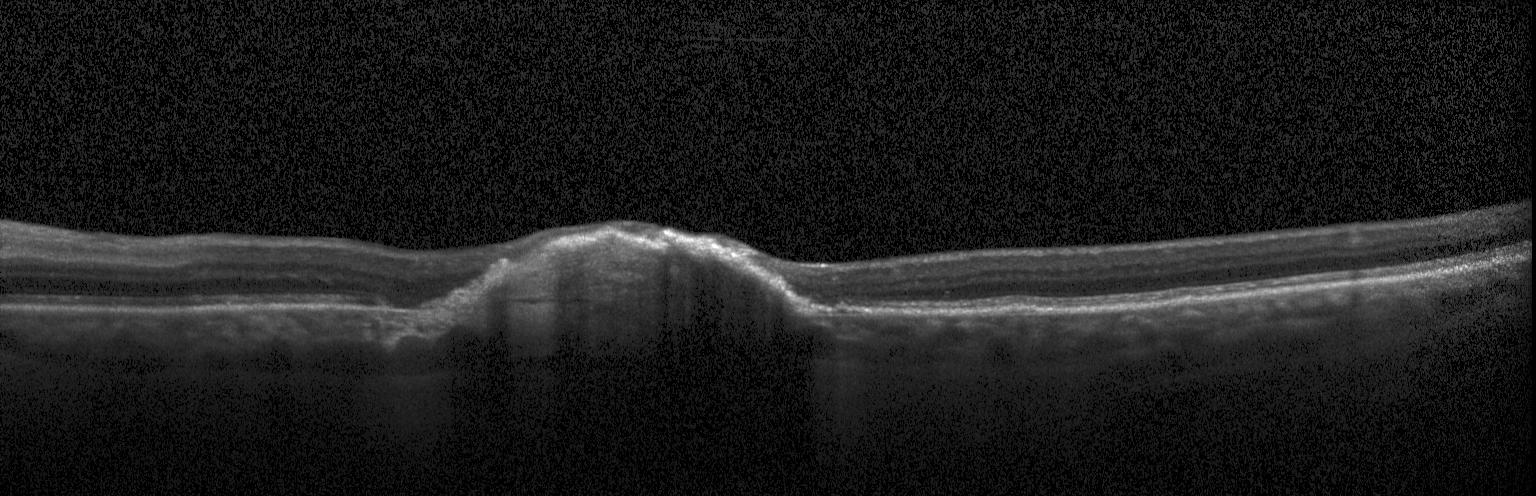

Instrument: Heidelberg Spectralis, through the macula, optical coherence tomography scan
Dx: choroidal neovascularization.